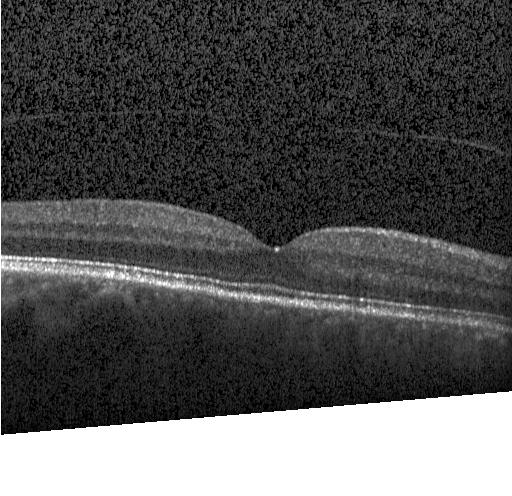 Impression: no evidence of choroidal neovascularization, diabetic macular edema, or drusen.